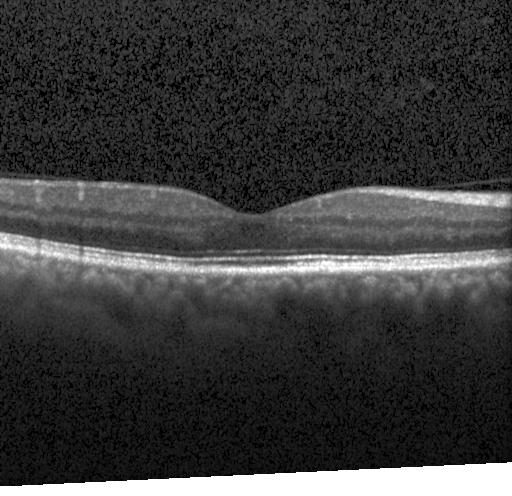 Heidelberg Spectralis OCT system. OCT B-scan
Assessment: no choroidal neovascularization, no diabetic macular edema, and no drusen.